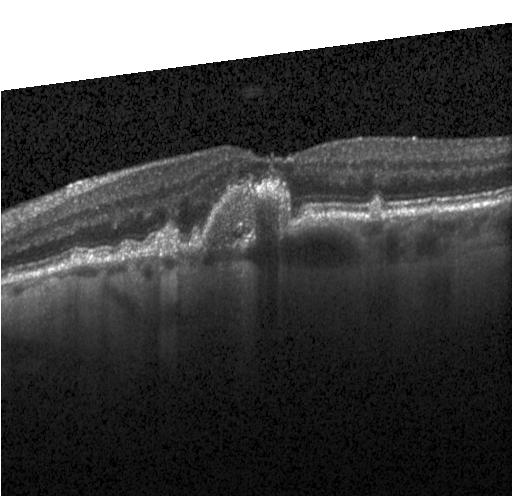

Optical coherence tomography B-scan · SD-OCT. Diagnosis: a choroidal neovascular membrane.